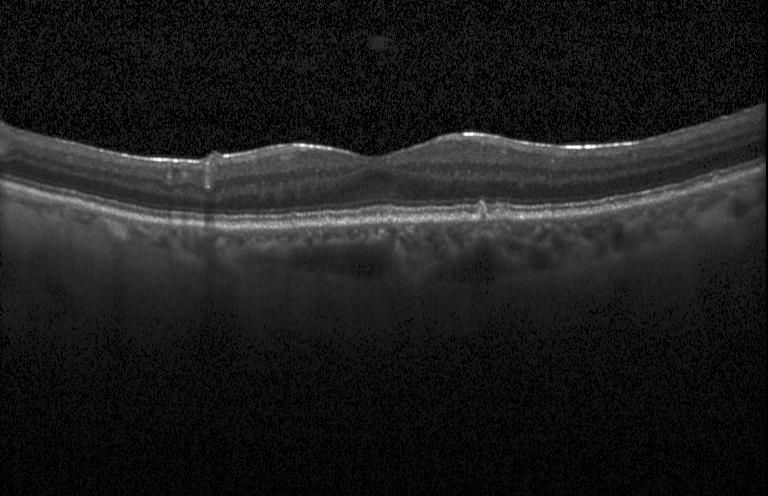

Impression: drusen.